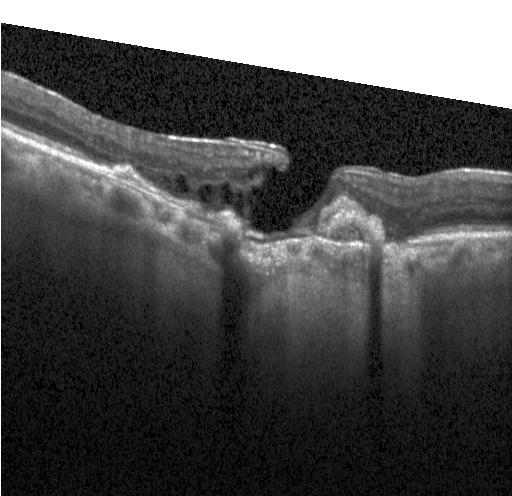
Horizontal scan through the fovea, optical coherence tomography scan — Diagnosis: choroidal neovascularization.